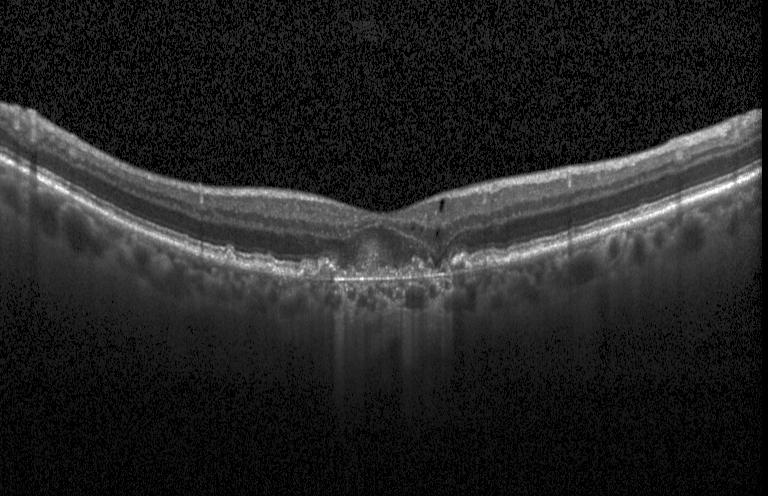

Finding: a choroidal neovascular membrane.